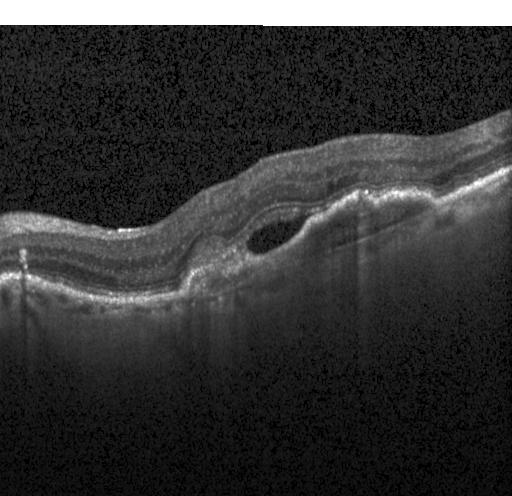

Macular scan. Optical coherence tomography B-scan — This B-scan demonstrates choroidal neovascularization (CNV).